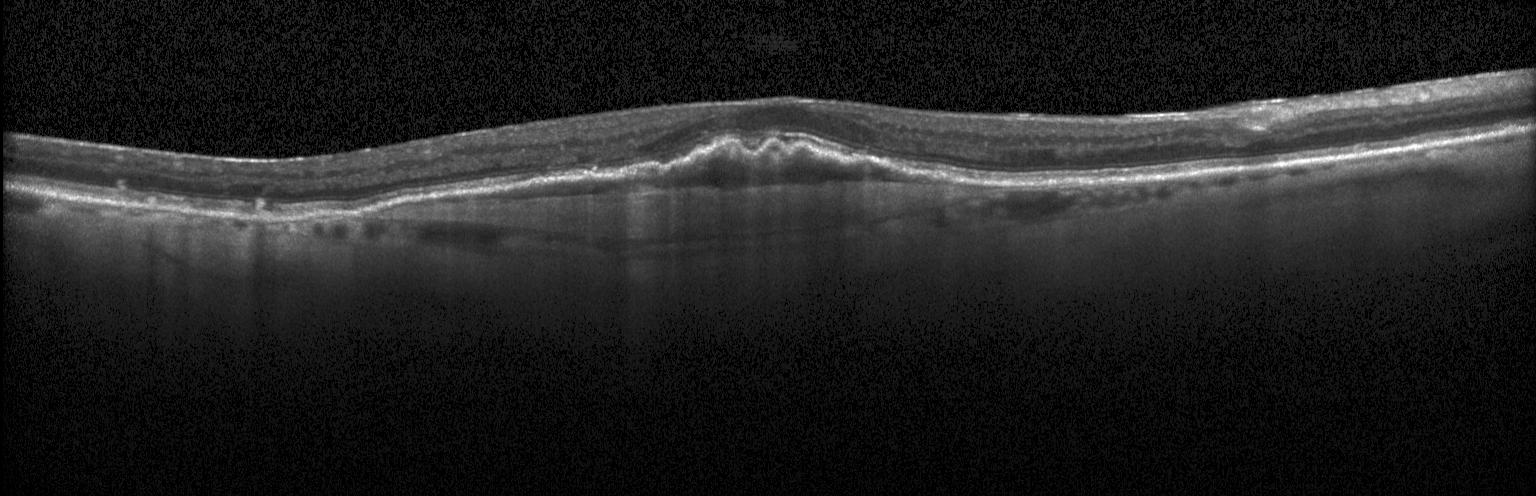

SD-OCT; optical coherence tomography scan; acquired on a Heidelberg Spectralis.
Dx: a choroidal neovascular membrane.